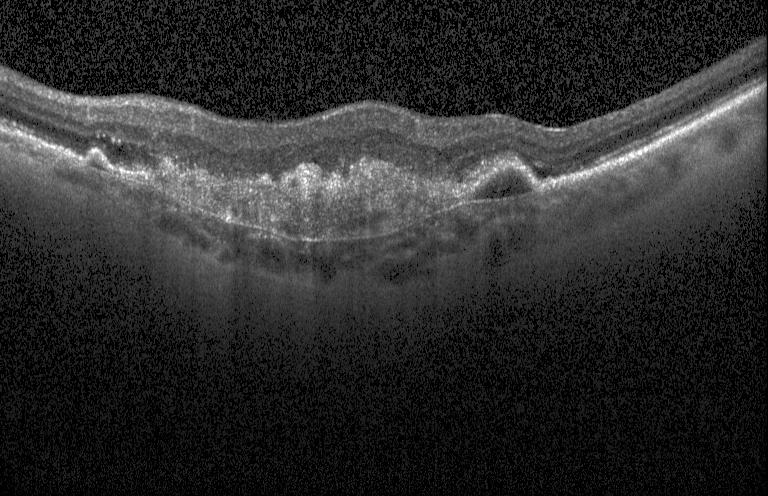
Centered on the fovea · Heidelberg Spectralis OCT system · retinal OCT cross-section
Finding: a choroidal neovascular membrane.